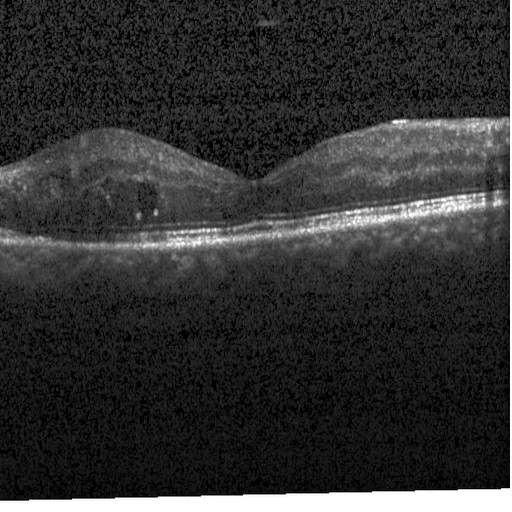 OCT scan showing diabetic macular edema (DME).